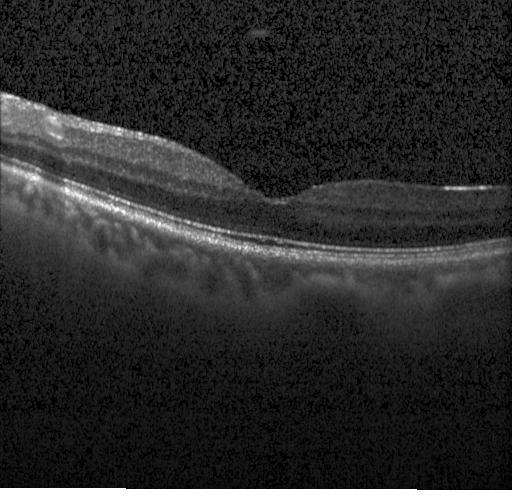
Dx: no CNV, no DME, and no drusen.